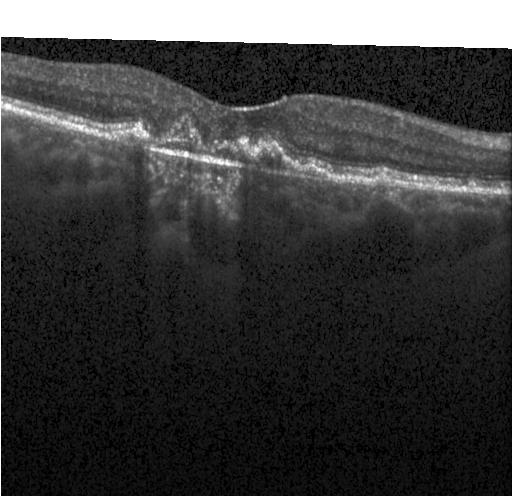 Horizontal scan through the fovea, retinal OCT B-scan, instrument: Heidelberg Spectralis, spectral-domain OCT — Finding: a choroidal neovascular membrane.